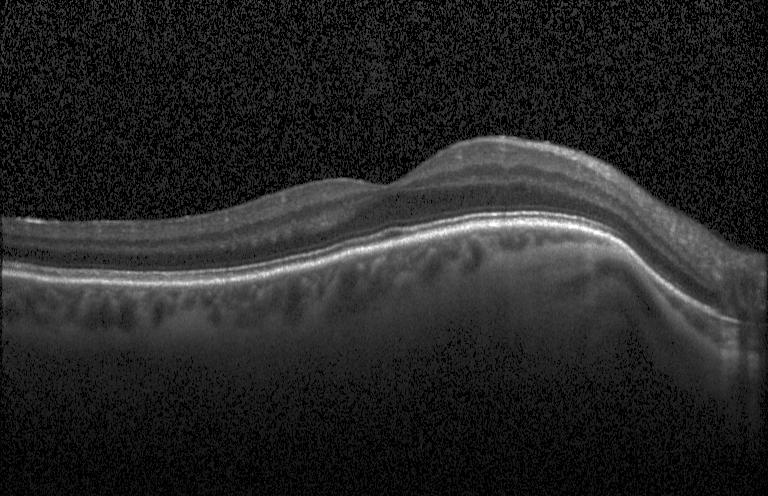

Spectral-domain OCT; optical coherence tomography B-scan; fovea-centered; instrument: Heidelberg Spectralis.
Assessment: no evidence of CNV, DME, or drusen.